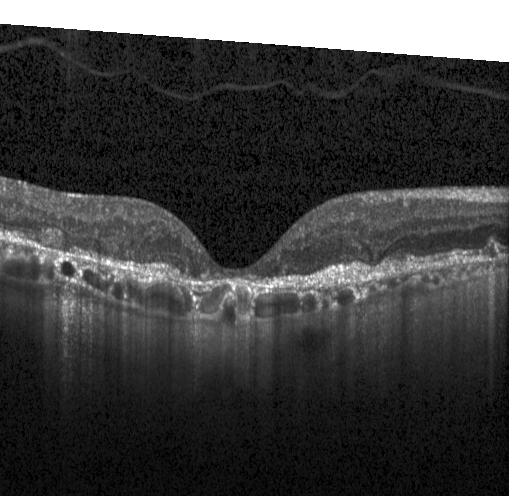 OCT B-scan showing a choroidal neovascular membrane.